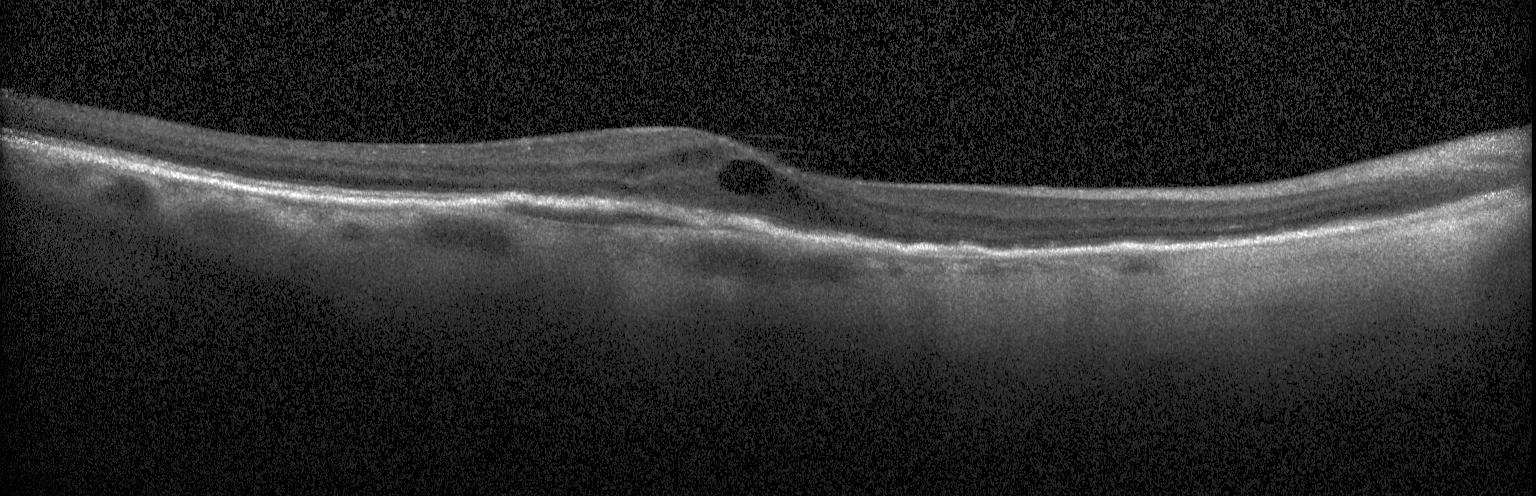 Diagnosis: CNV.